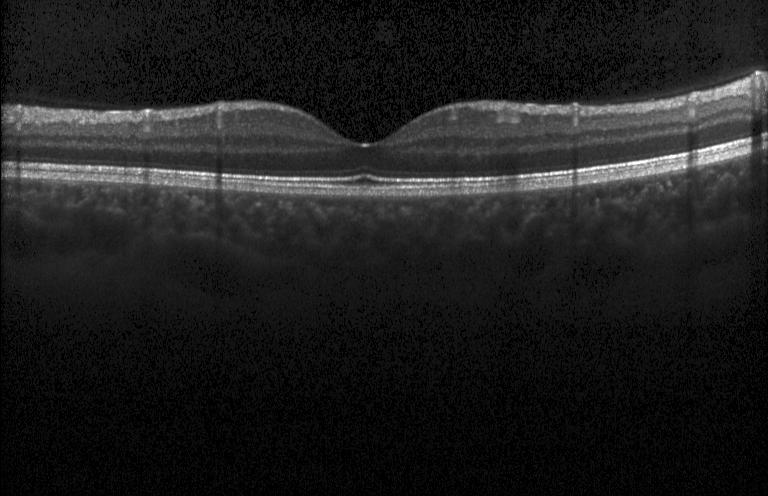 Finding: no evidence of choroidal neovascularization, diabetic macular edema, or drusen.